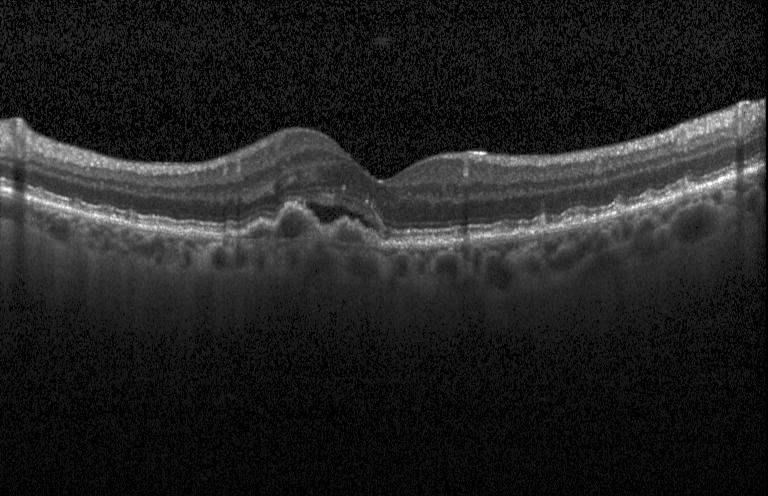

OCT line scan. SD-OCT. Acquired on a Heidelberg Spectralis. Centered on the fovea.
Macular OCT: a choroidal neovascular membrane.